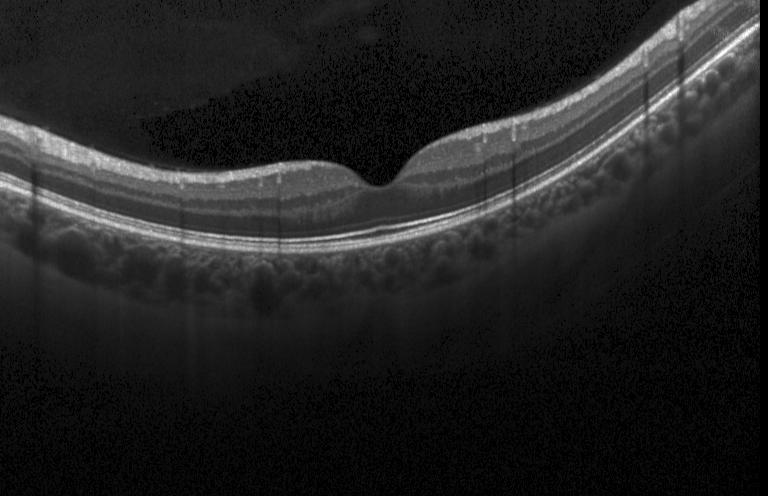
Heidelberg Spectralis, SD-OCT, macular scan, optical coherence tomography scan — The scan shows no evidence of choroidal neovascularization, diabetic macular edema, or drusen.